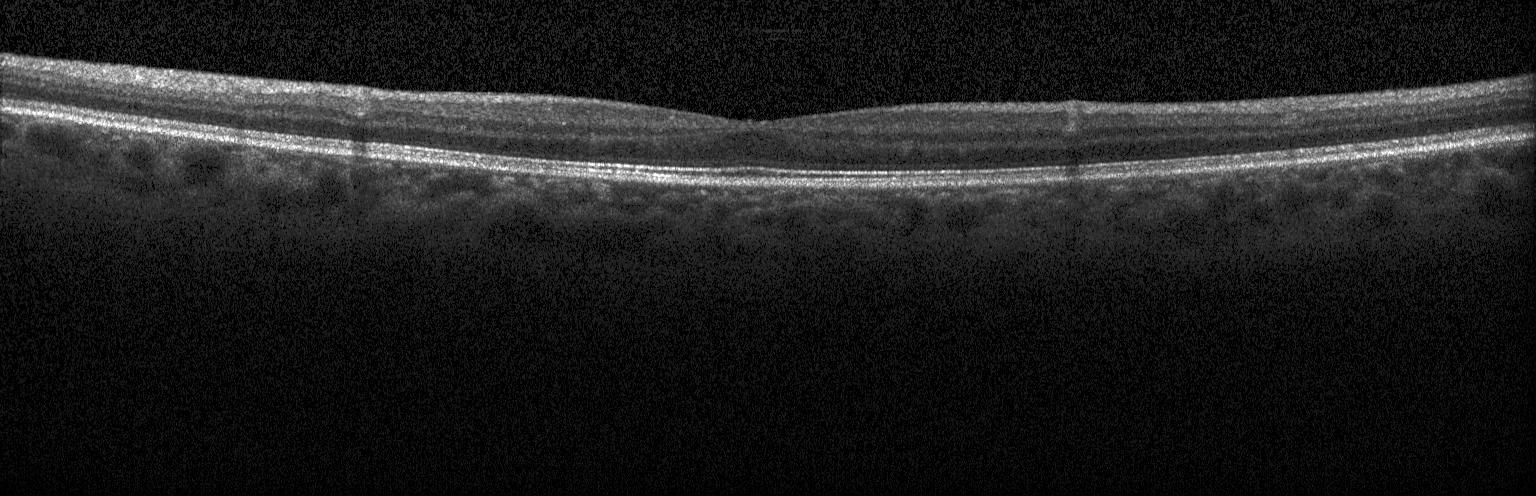

OCT B-scan. Finding: no choroidal neovascularization, diabetic macular edema, or drusen.